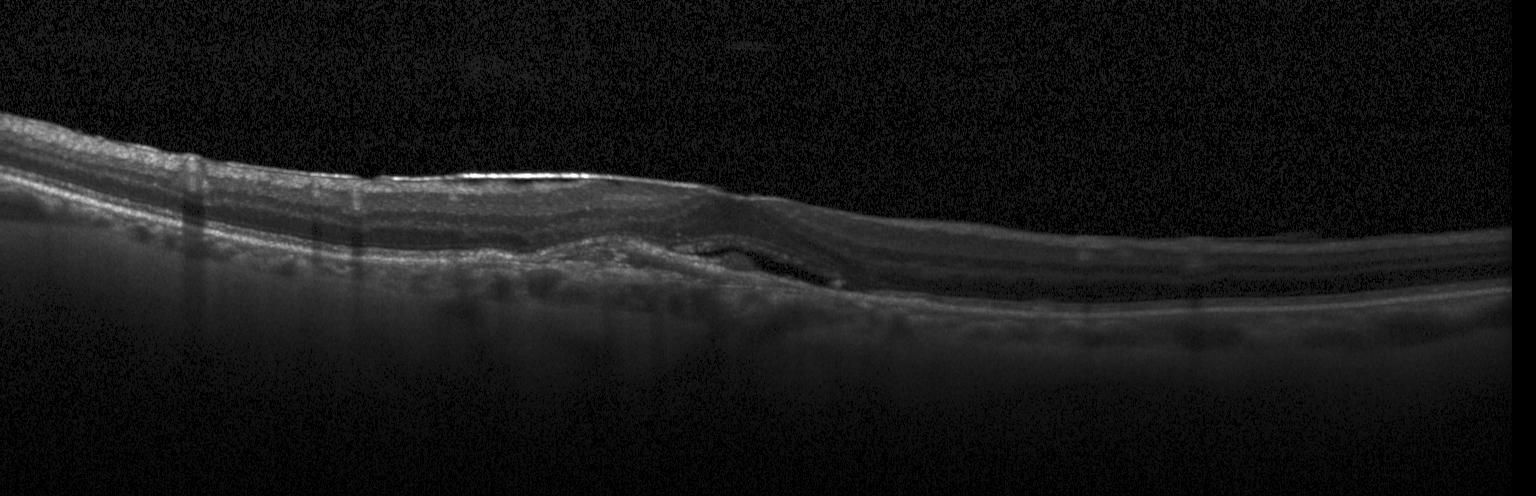

Optical coherence tomography B-scan — This B-scan demonstrates choroidal neovascularization.